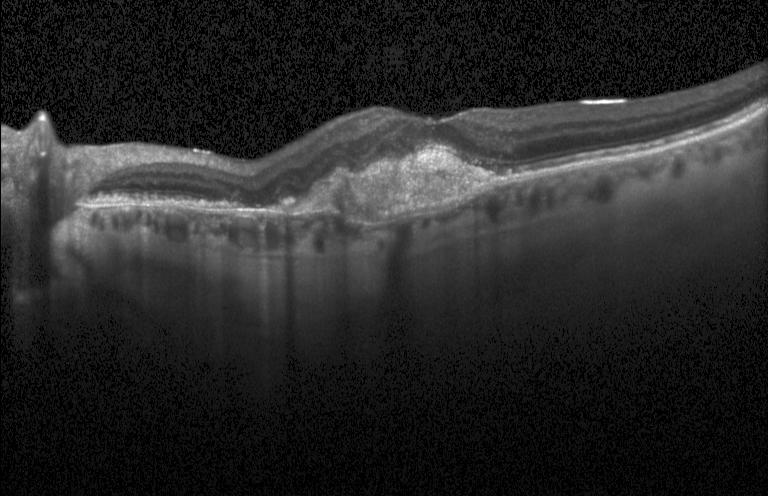 Spectral-domain optical coherence tomography. OCT B-scan — Macular OCT: CNV.